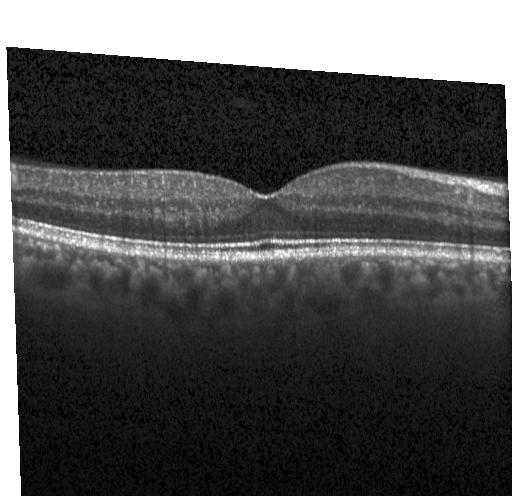

Impression: no CNV, no DME, and no drusen.